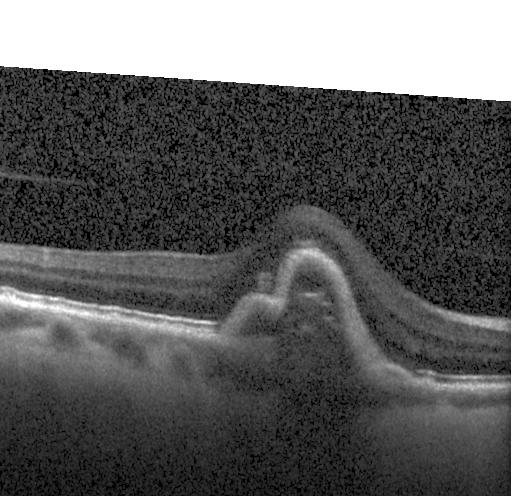 Heidelberg Spectralis OCT system. Spectral-domain optical coherence tomography. Retinal OCT B-scan — Assessment: CNV.